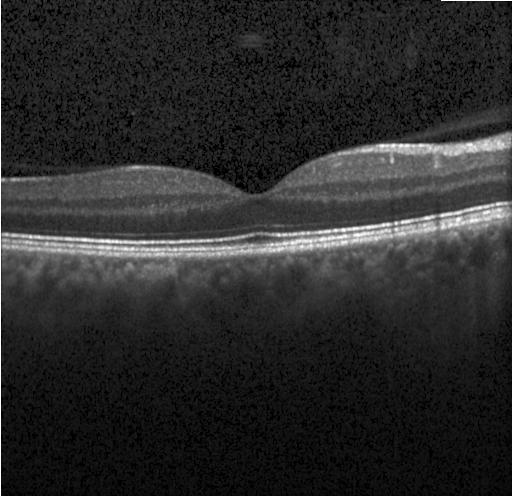
Finding: neither choroidal neovascularization, diabetic macular edema, nor drusen.